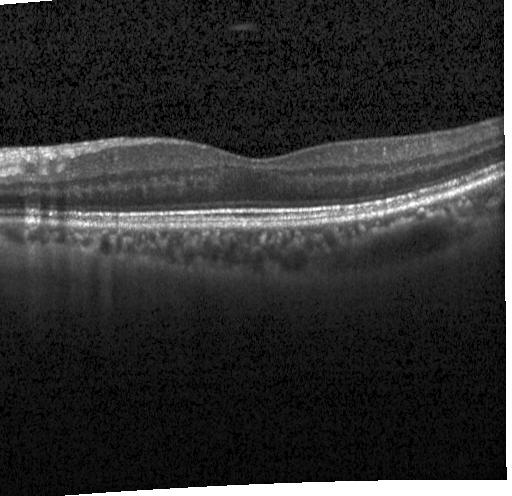 OCT B-scan. Horizontal scan through the fovea
Diagnosis: no choroidal neovascularization, no diabetic macular edema, and no drusen.